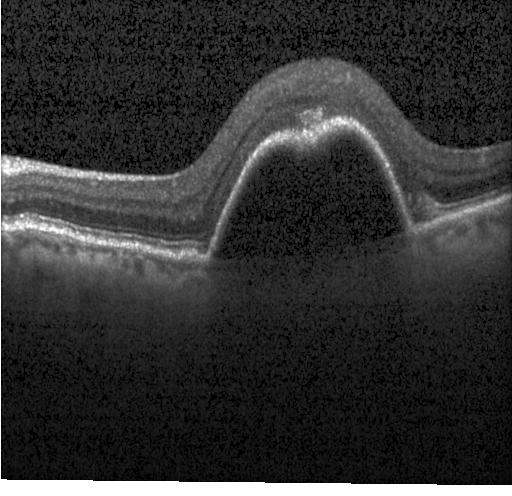
OCT finding: a choroidal neovascular membrane.